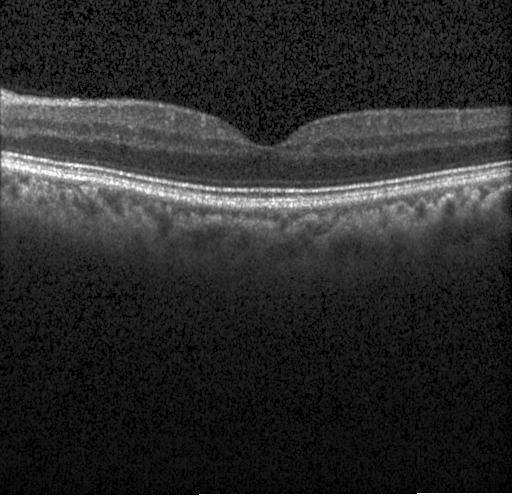

Retinal OCT cross-section.
Impression: no choroidal neovascularization, no diabetic macular edema, and no drusen.